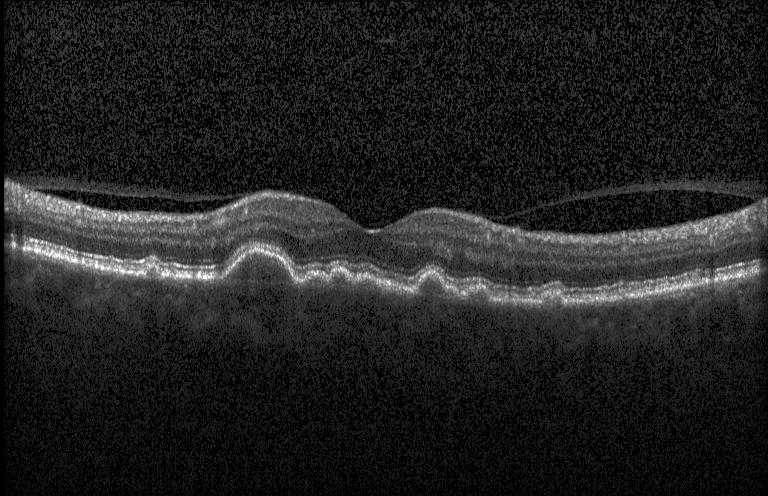
Optical coherence tomography B-scan · SD-OCT · horizontal scan through the fovea · acquired on a Heidelberg Spectralis — Impression: multiple drusen.